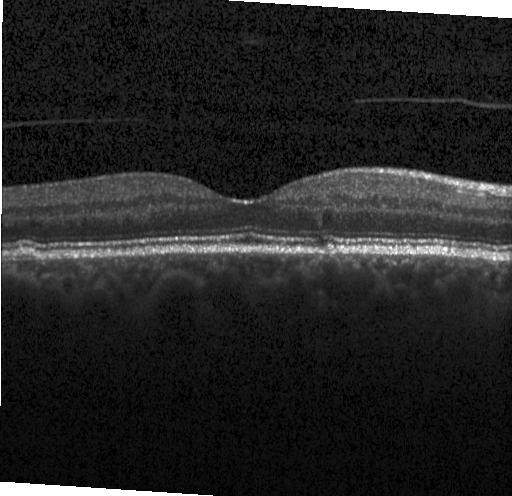

Heidelberg Spectralis OCT system. Spectral-domain OCT. OCT line scan. Macular scan
Impression: drusen.